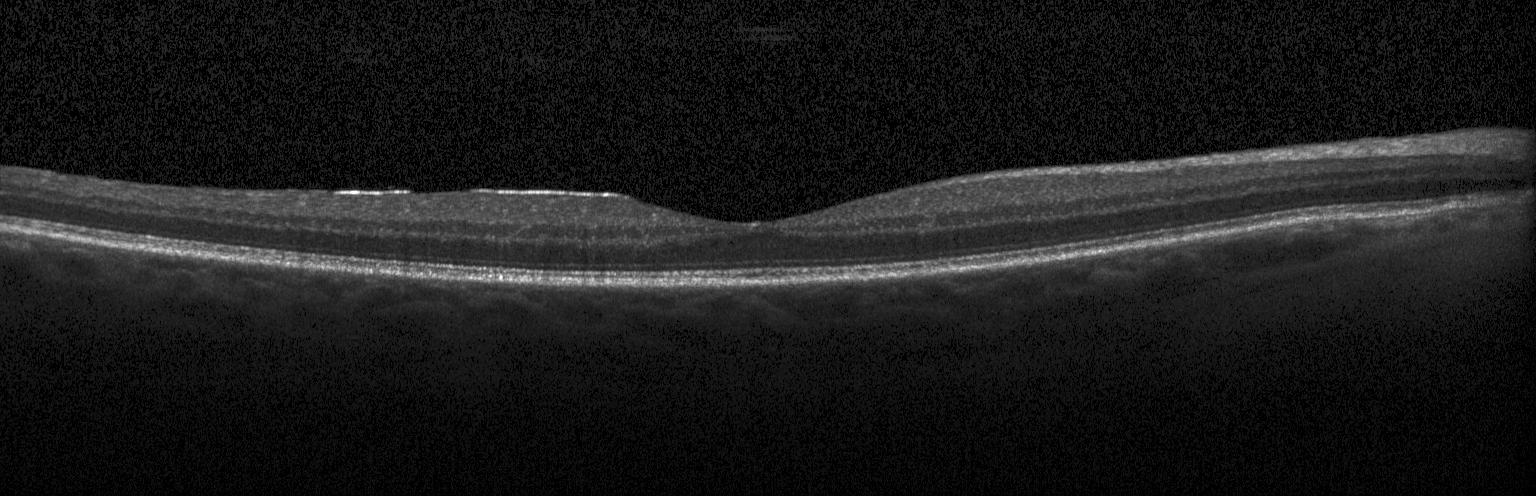 Macular scan; acquired on a Heidelberg Spectralis; retinal OCT cross-section; spectral-domain OCT
Diagnosis: no evidence of CNV, DME, or drusen.